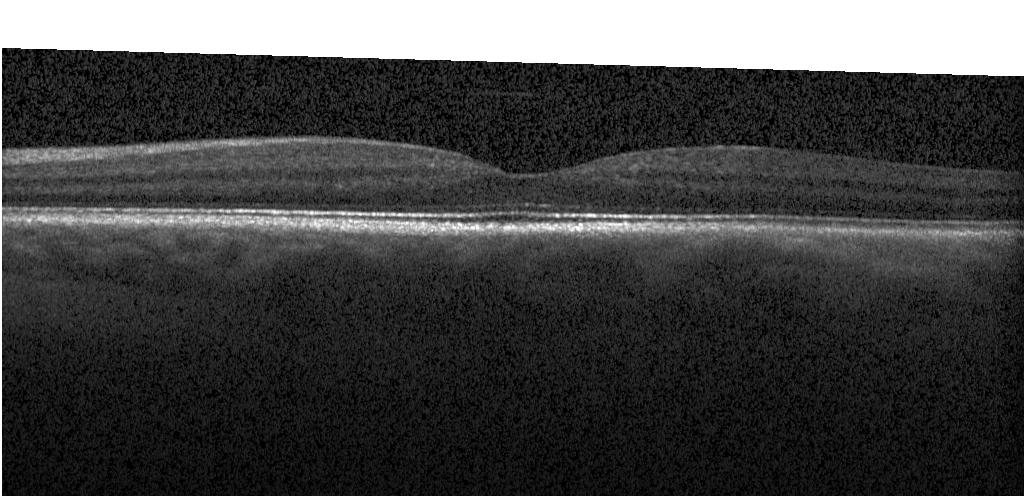
Assessment: no evidence of choroidal neovascularization, diabetic macular edema, or drusen.